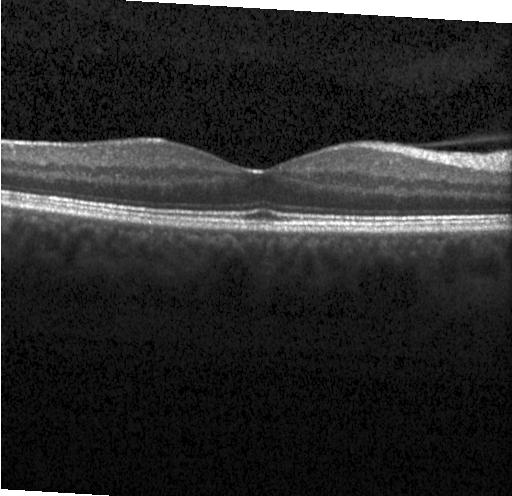
OCT B-scan, spectral-domain OCT. No evidence of choroidal neovascularization, diabetic macular edema, or drusen.